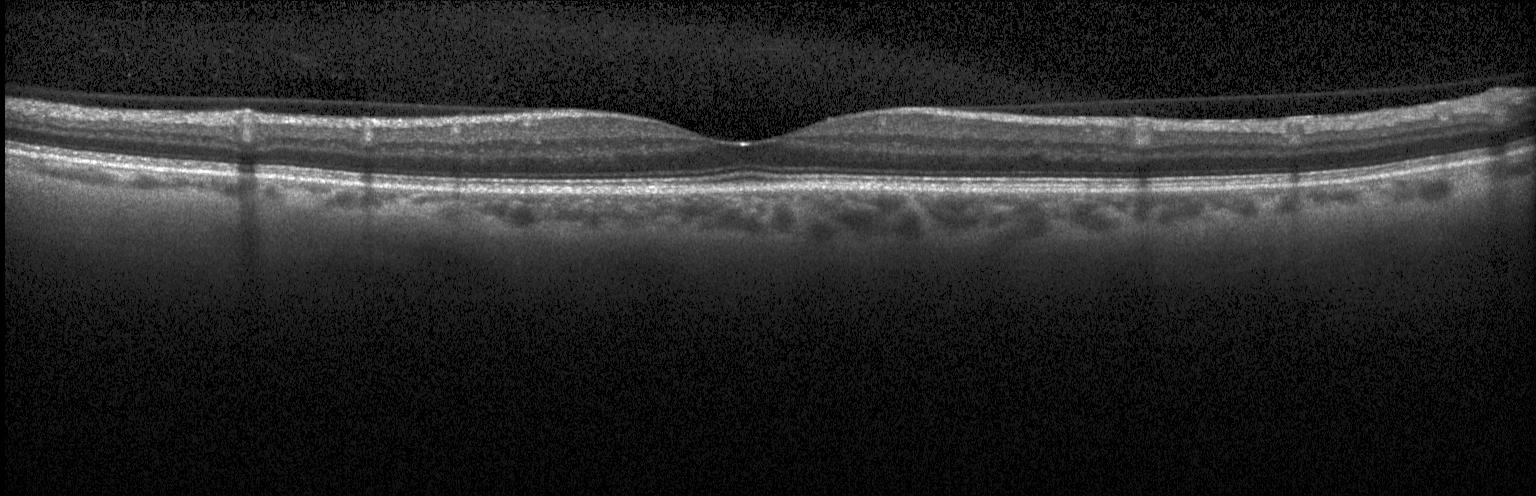
OCT scan showing no choroidal neovascularization, no diabetic macular edema, and no drusen.